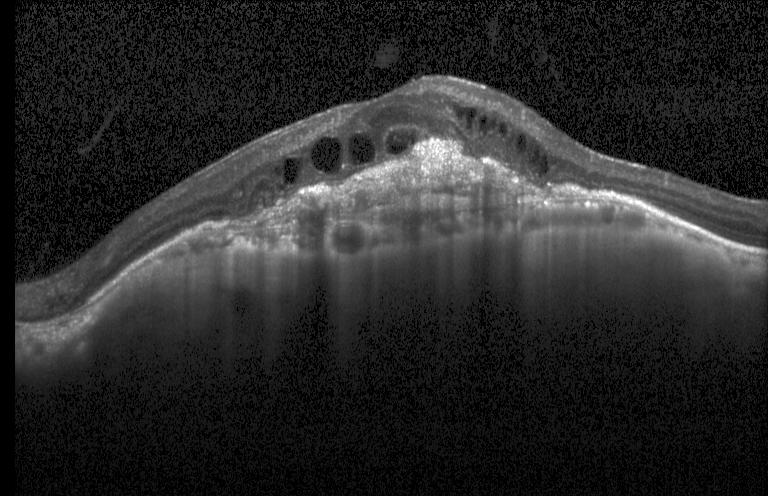

Diagnosis: a choroidal neovascular membrane.